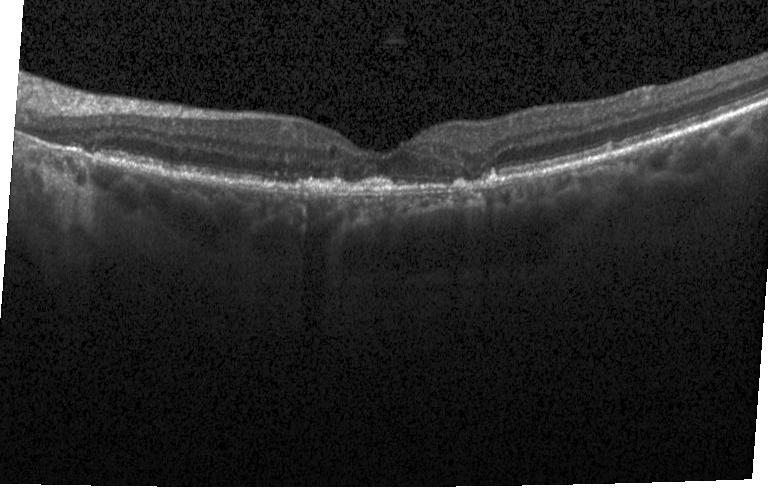 OCT line scan — Assessment: a choroidal neovascular membrane.